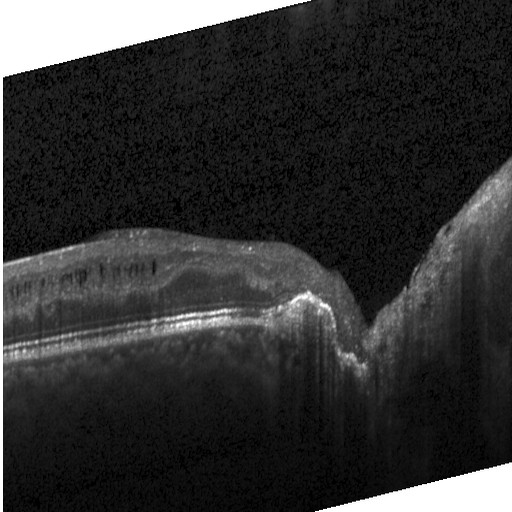

OCT line scan
This B-scan demonstrates diabetic macular edema (DME).